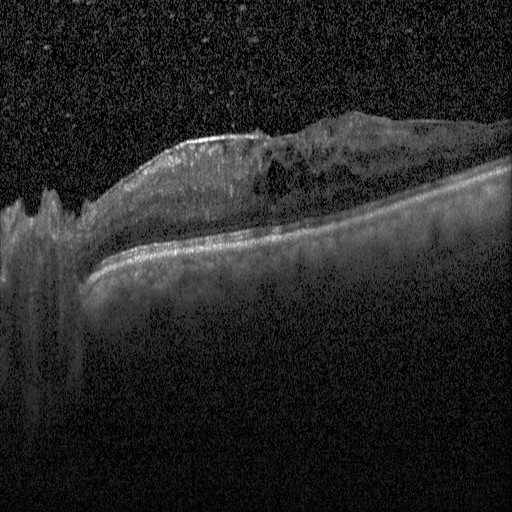

Optical coherence tomography B-scan; Heidelberg Spectralis OCT system
Diagnosis: diabetic macular edema.